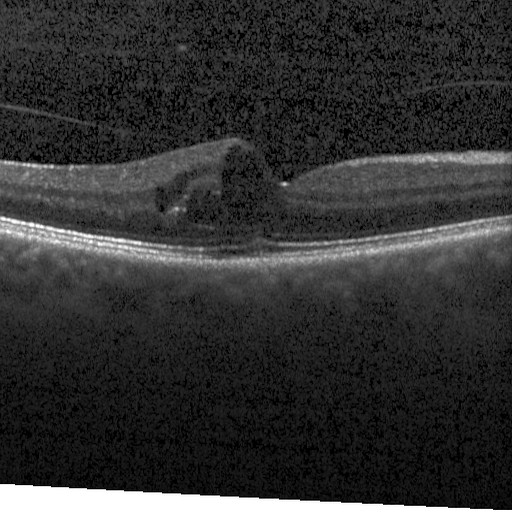

Retinal OCT B-scan, Heidelberg Spectralis, fovea-centered. This B-scan demonstrates diabetic macular edema (DME).